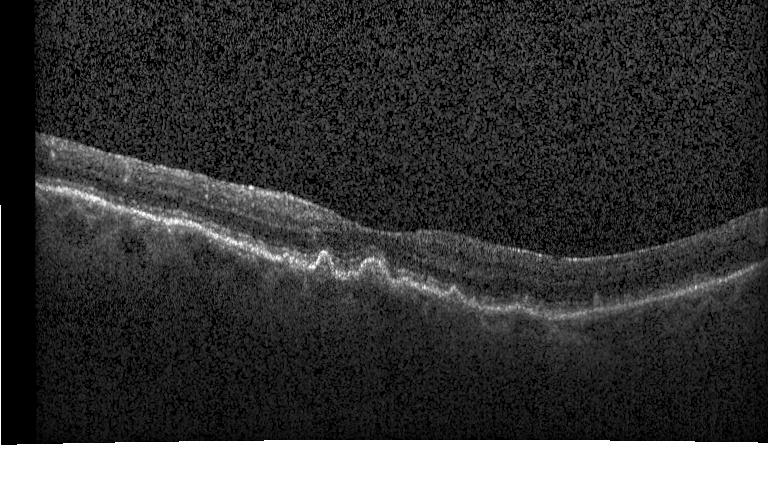 Spectral-domain optical coherence tomography; horizontal scan through the fovea; optical coherence tomography scan; instrument: Heidelberg Spectralis — Diagnosis: multiple drusen.